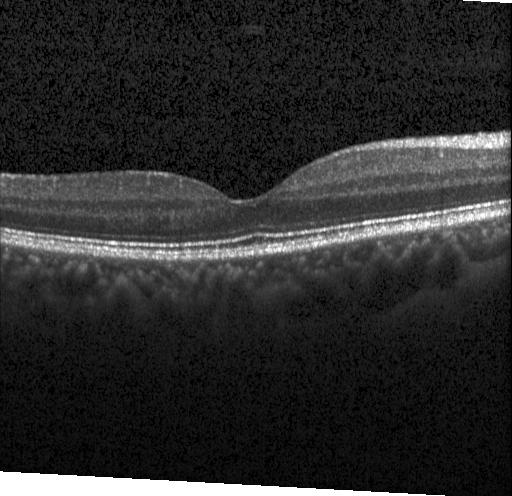
Retinal OCT B-scan.
Assessment: no CNV, no DME, and no drusen.